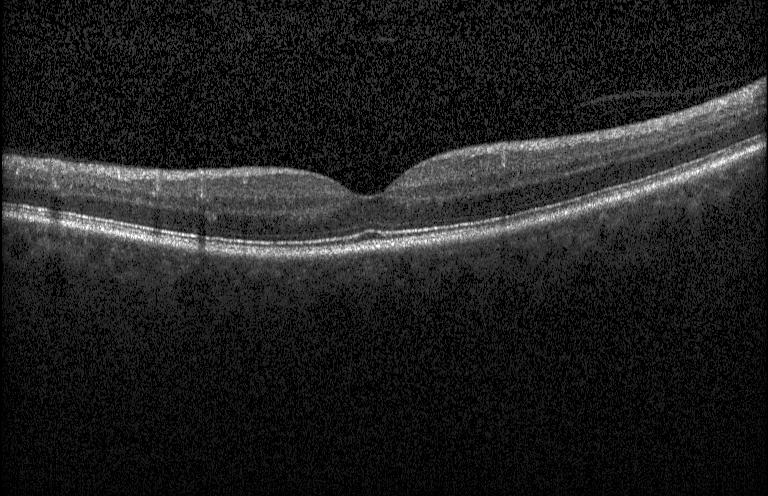 Optical coherence tomography scan, spectral-domain optical coherence tomography, acquired on a Heidelberg Spectralis.
Impression: no choroidal neovascularization, diabetic macular edema, or drusen.